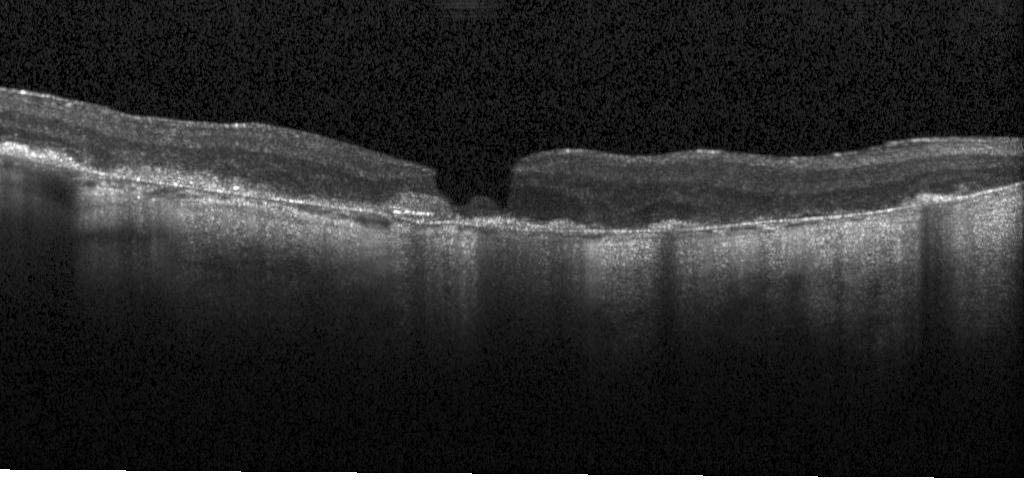 Retinal OCT cross-section
OCT finding: a choroidal neovascular membrane.